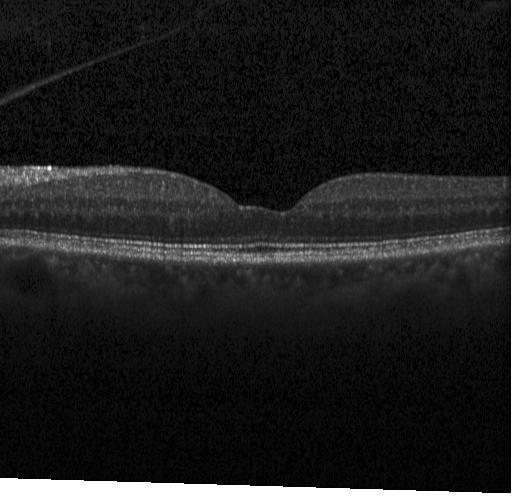
Centered on the fovea. OCT line scan. Assessment: no evidence of choroidal neovascularization, diabetic macular edema, or drusen.